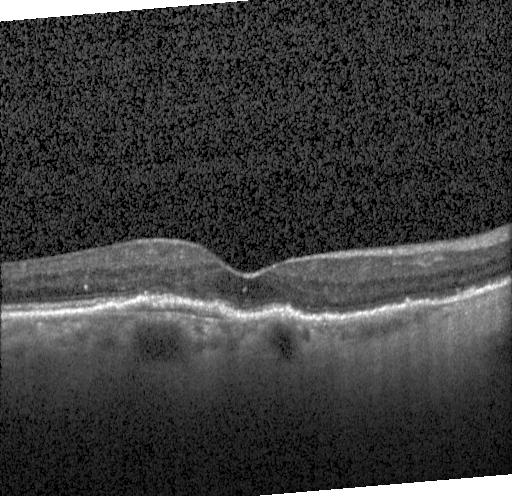

Optical coherence tomography B-scan.
Impression: a choroidal neovascular membrane.